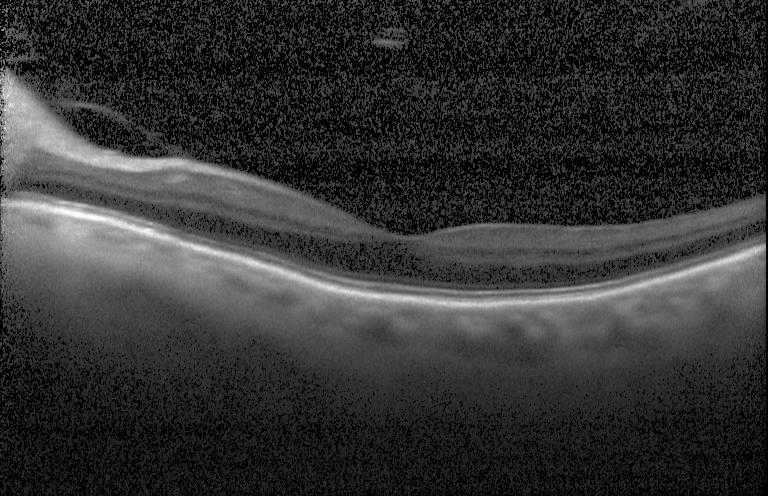
Optical coherence tomography scan. Diagnosis: neither choroidal neovascularization, diabetic macular edema, nor drusen.